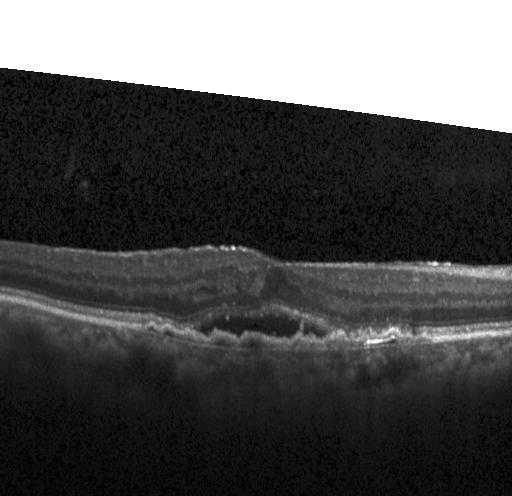

OCT line scan; Heidelberg Spectralis. Diagnosis: a choroidal neovascular membrane.